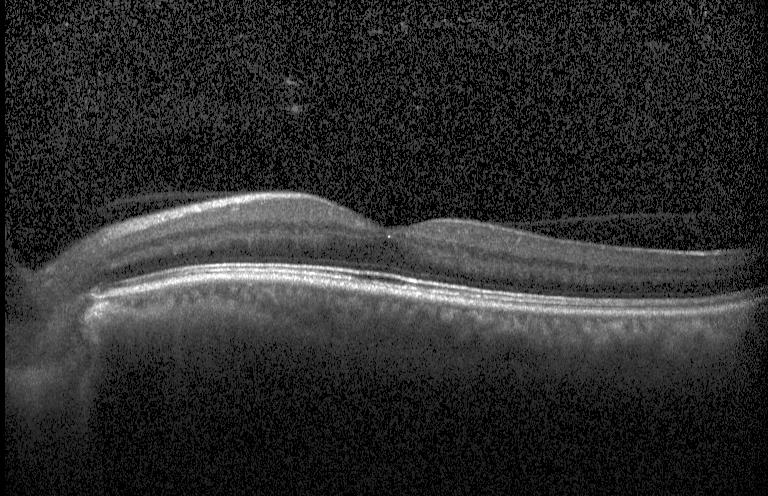
OCT B-scan showing no choroidal neovascularization, diabetic macular edema, or drusen.